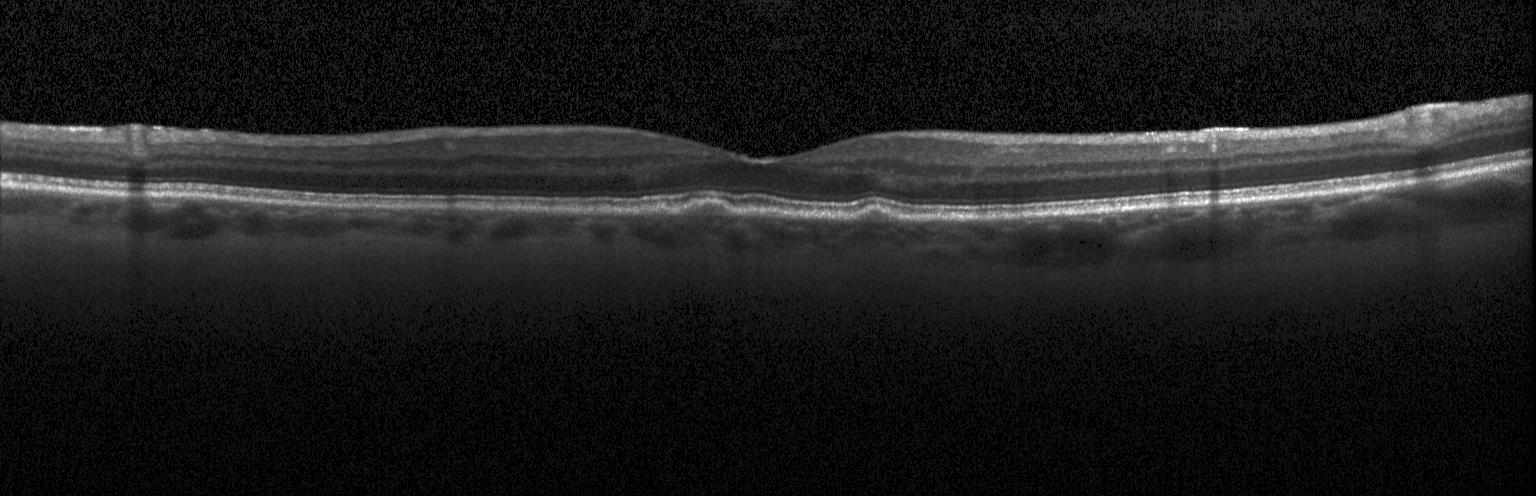 Spectral-domain OCT B-scan: drusen.